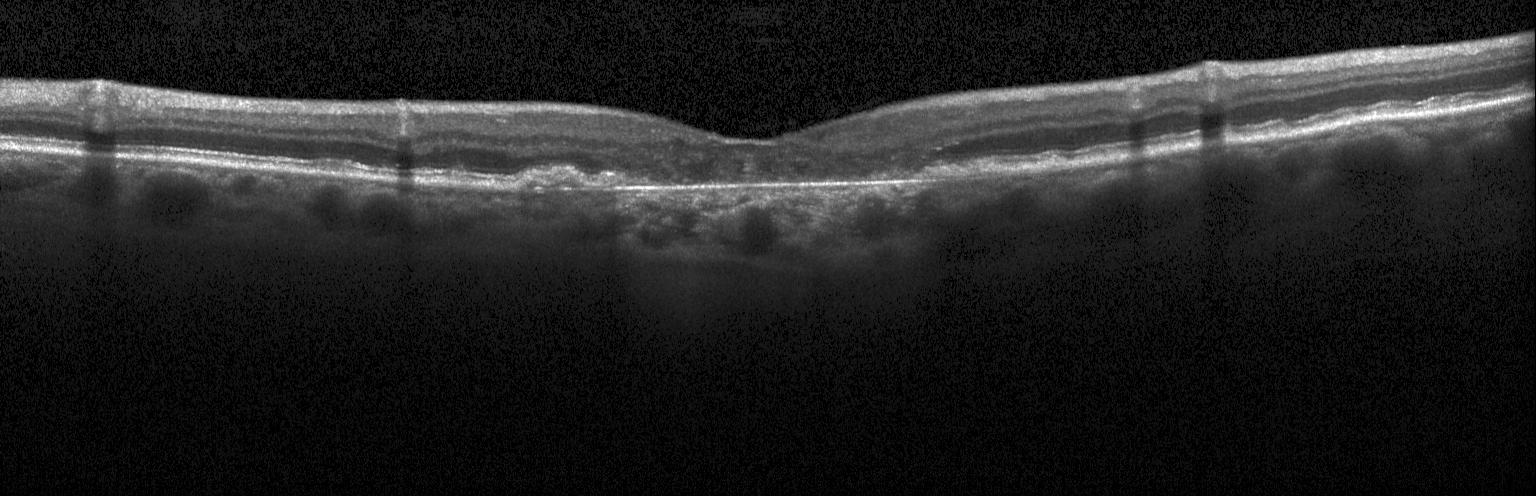 Acquired on a Heidelberg Spectralis; optical coherence tomography B-scan.
The scan shows CNV.